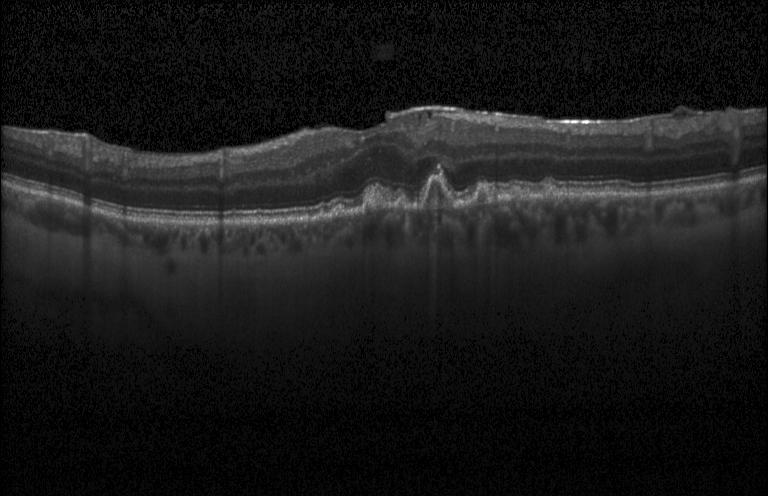
OCT finding: sub-RPE drusenoid deposits.